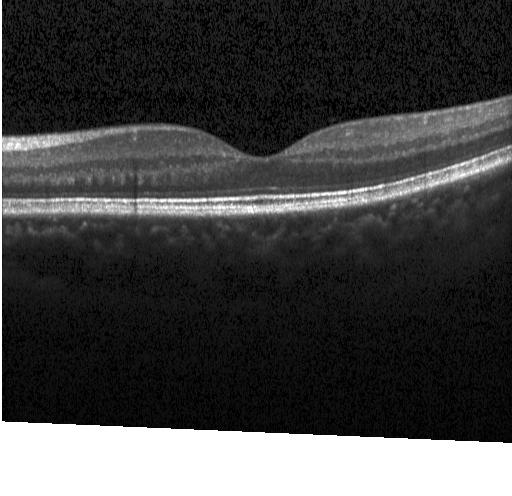 Finding: neither choroidal neovascularization, diabetic macular edema, nor drusen.